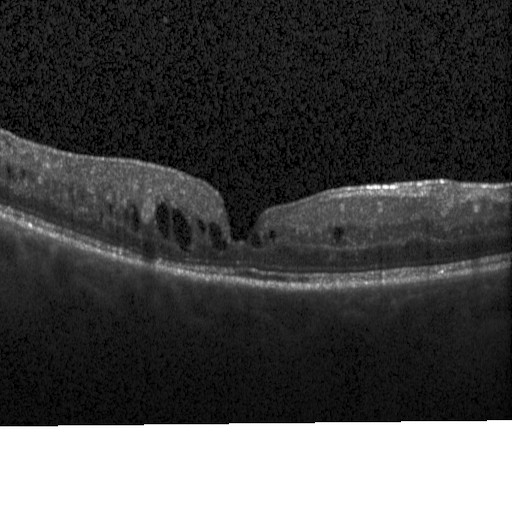 Through the macula. Spectral-domain optical coherence tomography. Heidelberg Spectralis OCT system. Optical coherence tomography scan
OCT finding: diabetic macular edema.